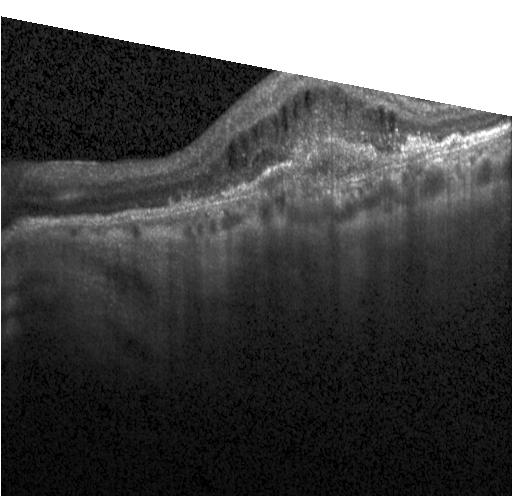

Diagnosis: CNV.